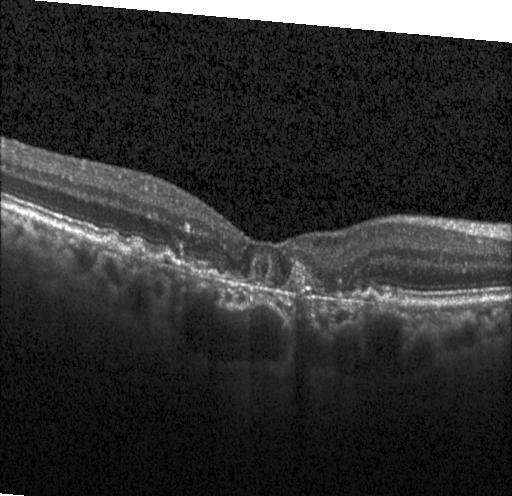

Through the macula. OCT B-scan. Heidelberg Spectralis OCT system. SD-OCT.
OCT finding: choroidal neovascularization (CNV).